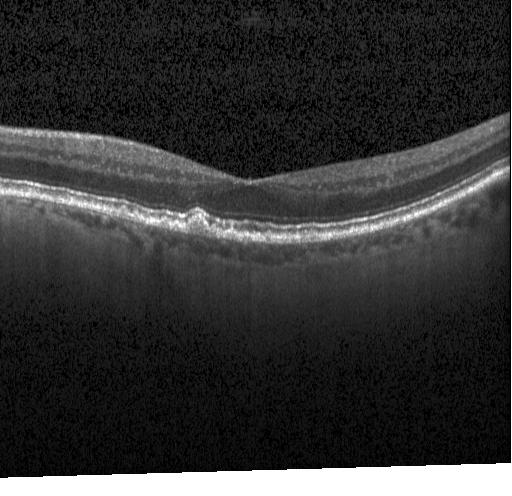 Optical coherence tomography B-scan.
Sub-RPE drusenoid deposits.